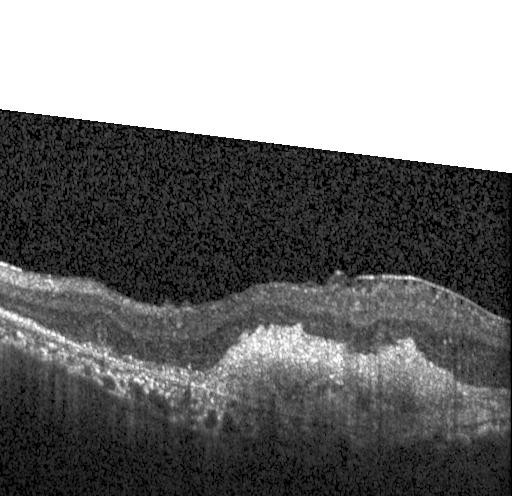 Spectral-domain OCT B-scan: choroidal neovascularization (CNV).